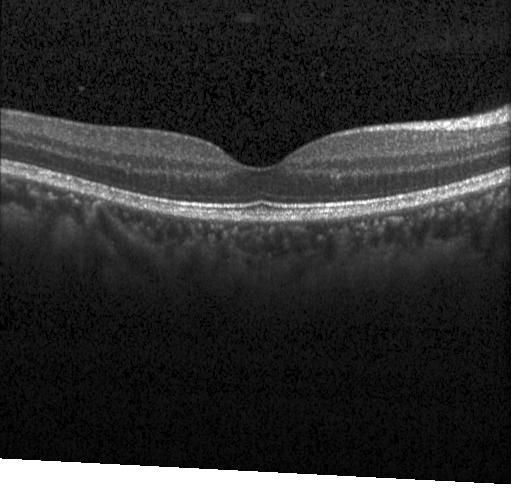

Heidelberg Spectralis OCT system, retinal OCT cross-section — No evidence of choroidal neovascularization, diabetic macular edema, or drusen.